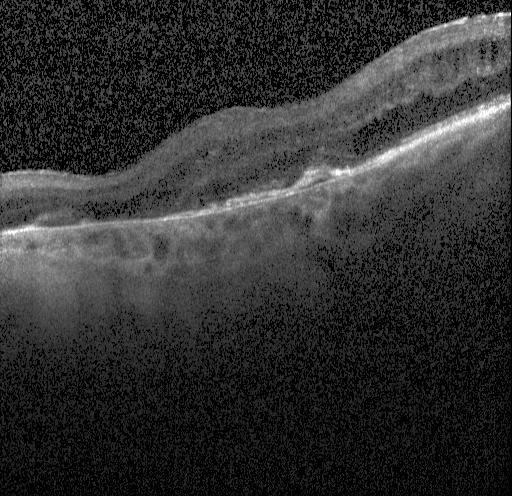
Retinal OCT cross-section, spectral-domain OCT, horizontal scan through the fovea.
Assessment: choroidal neovascularization.